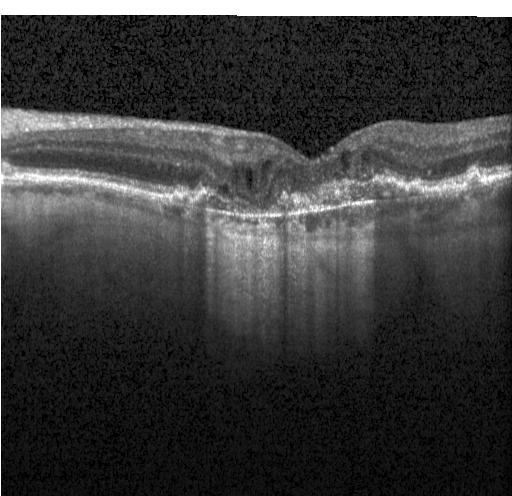
SD-OCT · OCT line scan · Heidelberg Spectralis
OCT finding: choroidal neovascularization (CNV).